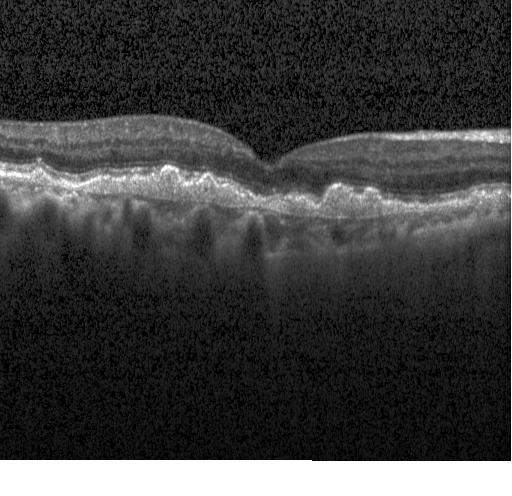

OCT finding: a choroidal neovascular membrane.